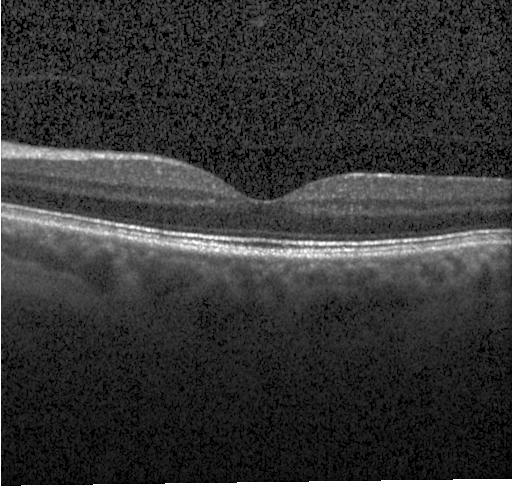 Fovea-centered; spectral-domain OCT; instrument: Heidelberg Spectralis; optical coherence tomography scan
Impression: neither choroidal neovascularization, diabetic macular edema, nor drusen.